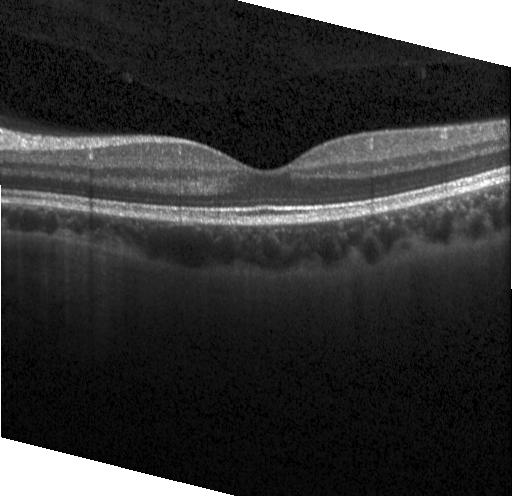

Impression: no evidence of CNV, DME, or drusen.